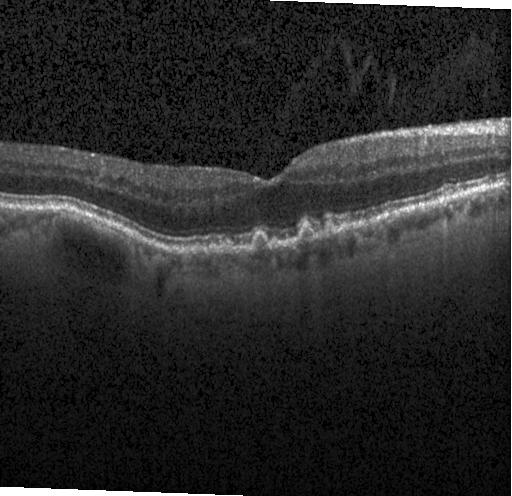
This B-scan demonstrates multiple drusen.